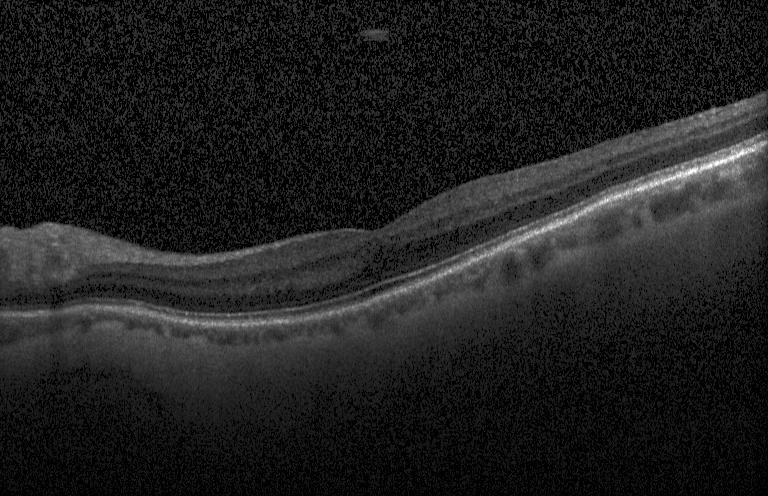 No CNV, DME, or drusen.